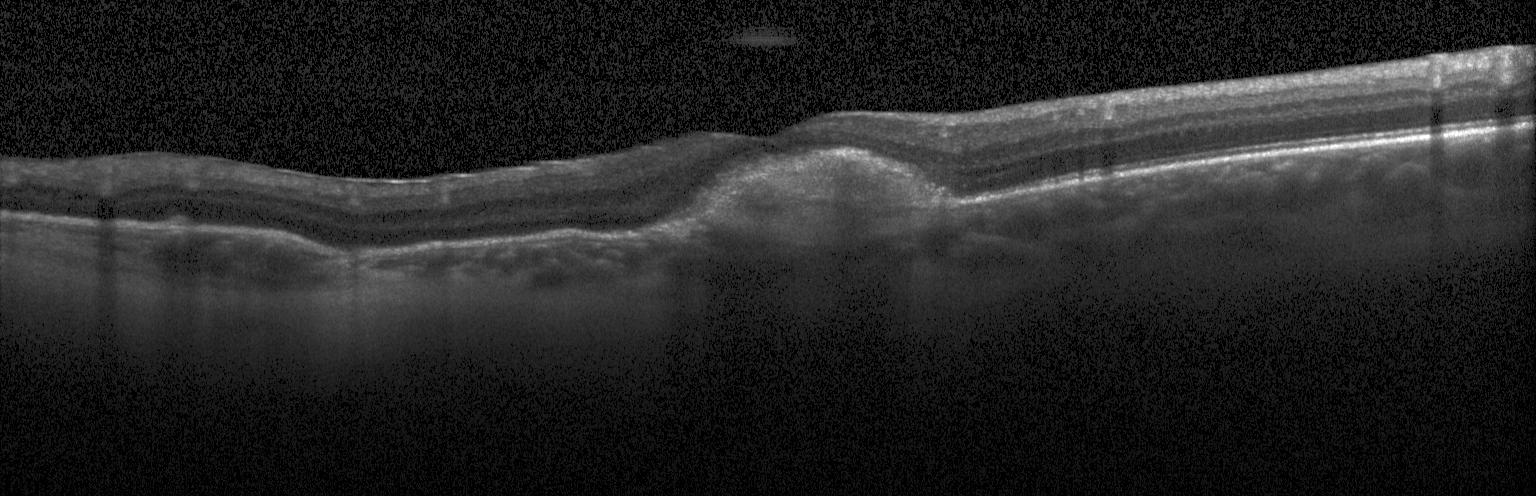 Choroidal neovascularization.